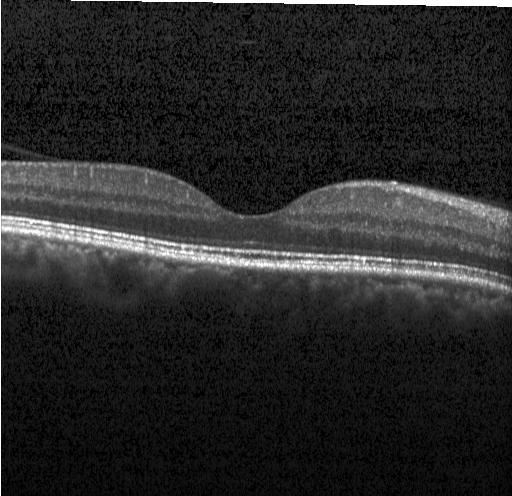
Finding: no evidence of choroidal neovascularization, diabetic macular edema, or drusen.